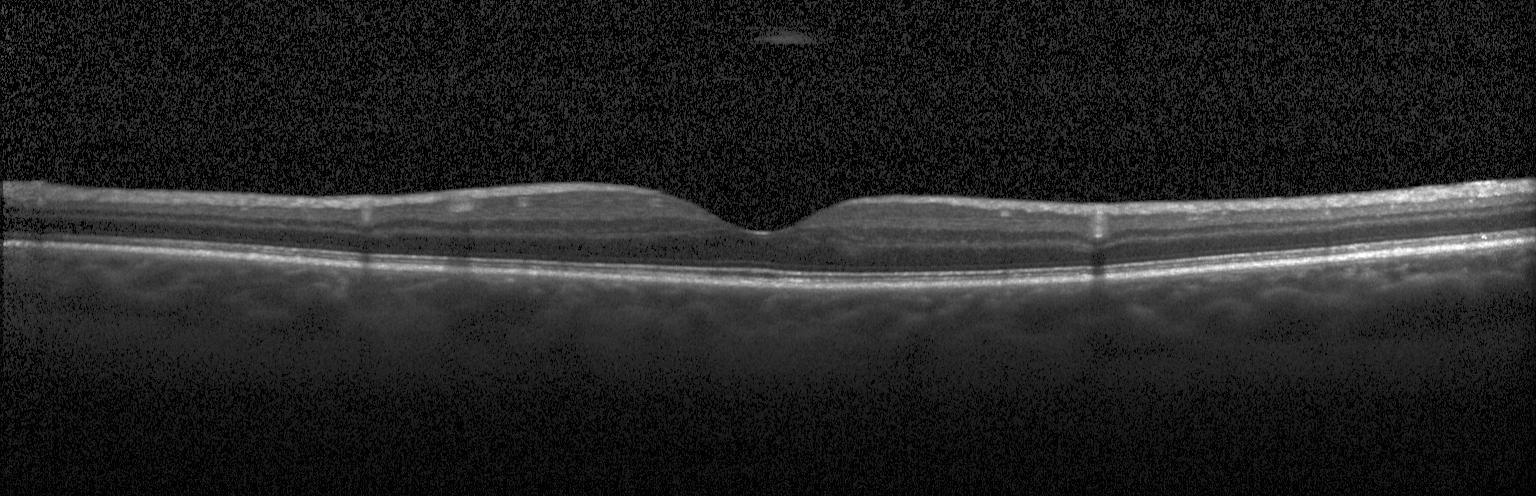 Diagnosis: neither choroidal neovascularization, diabetic macular edema, nor drusen.